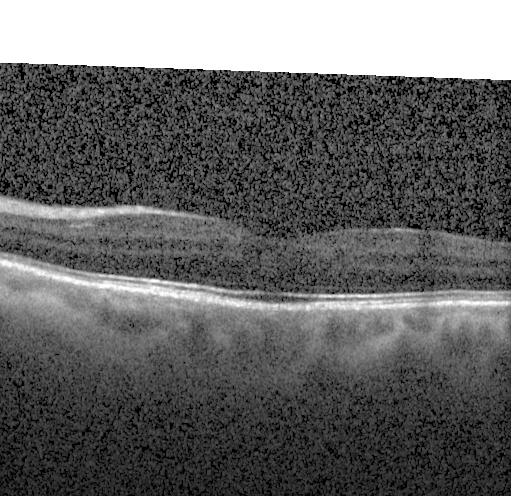
Assessment: no evidence of choroidal neovascularization, diabetic macular edema, or drusen.